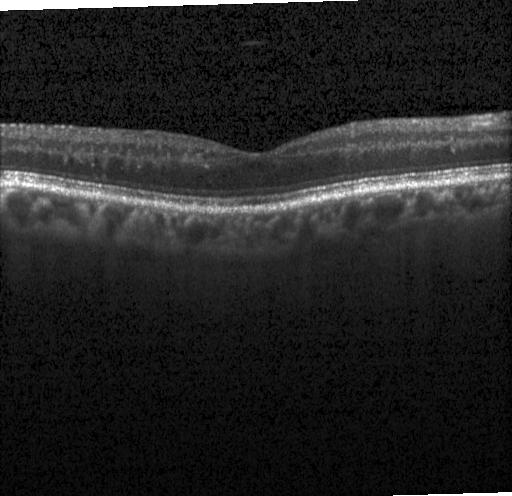 Spectral-domain optical coherence tomography. Heidelberg Spectralis. Optical coherence tomography B-scan — Macular OCT: no evidence of CNV, DME, or drusen.